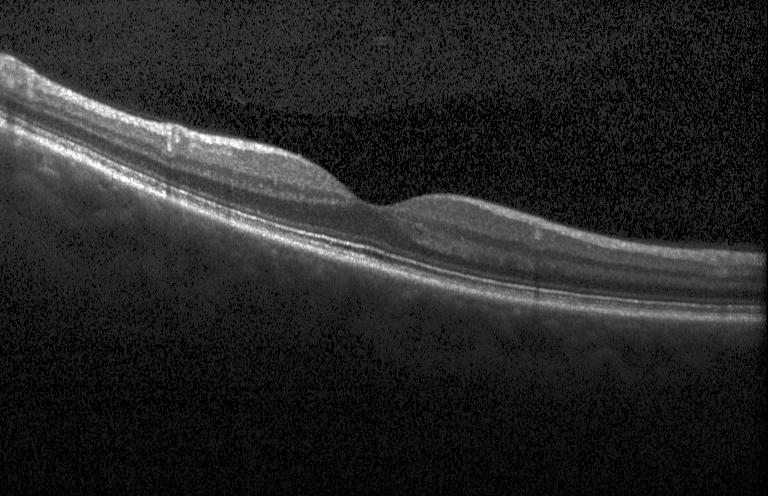
Optical coherence tomography B-scan · centered on the fovea · Heidelberg Spectralis OCT system · spectral-domain optical coherence tomography.
Dx: no choroidal neovascularization, diabetic macular edema, or drusen.